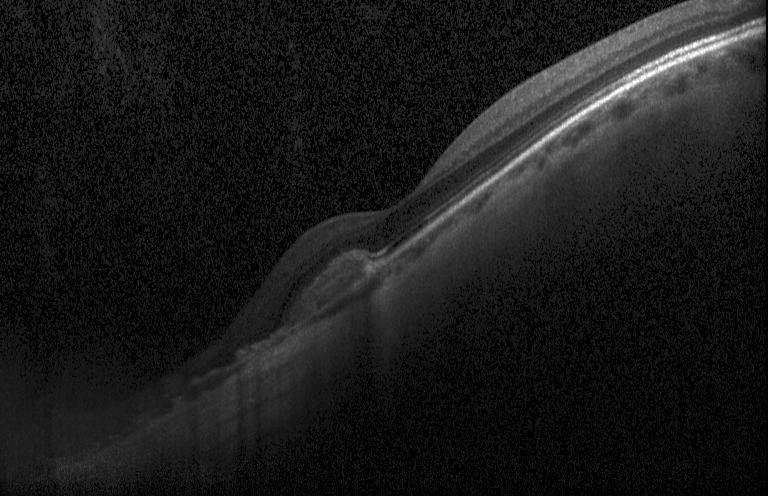 Spectral-domain optical coherence tomography. Horizontal scan through the fovea. OCT B-scan.
Impression: choroidal neovascularization (CNV).